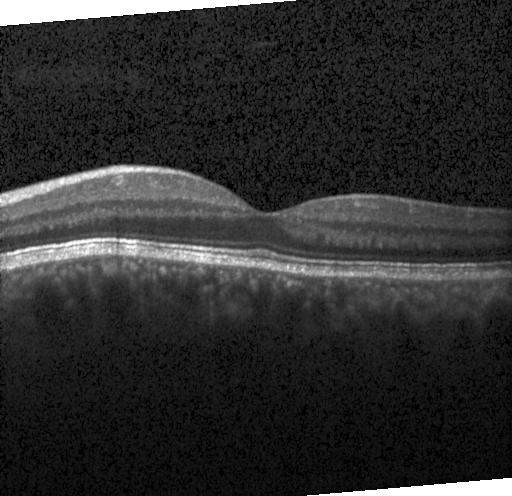
Diagnosis: no evidence of choroidal neovascularization, diabetic macular edema, or drusen.